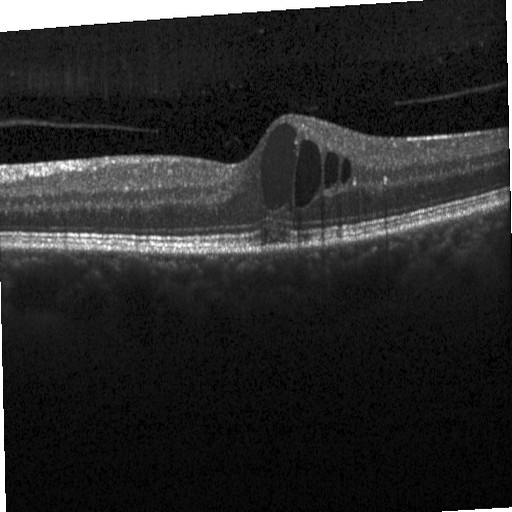 OCT B-scan, fovea-centered — Impression: DME.